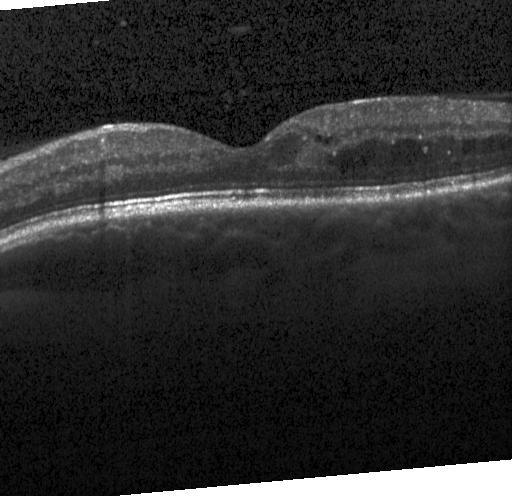 OCT B-scan · centered on the fovea · spectral-domain OCT — Assessment: diabetic macular edema.